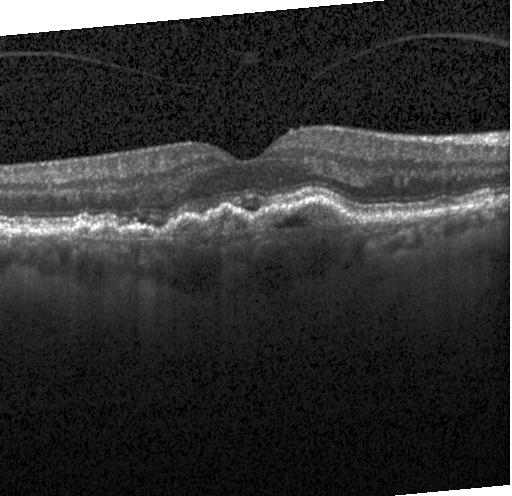
OCT B-scan; SD-OCT; horizontal scan through the fovea
Impression: choroidal neovascularization.